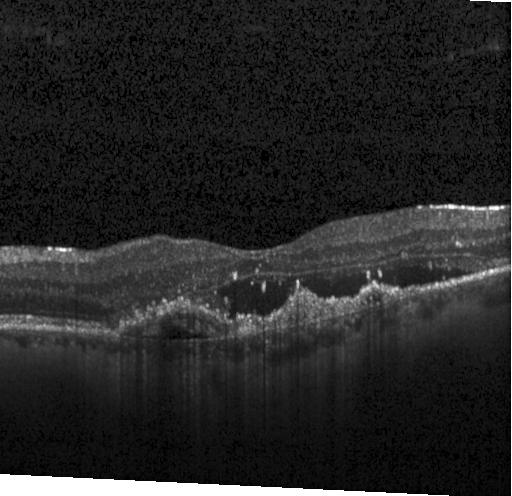
Diagnosis: CNV.